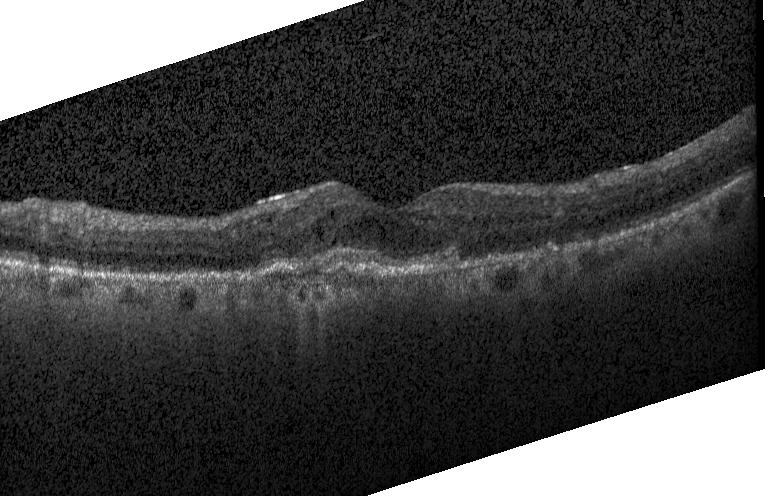

Retinal OCT B-scan — This B-scan demonstrates a choroidal neovascular membrane.